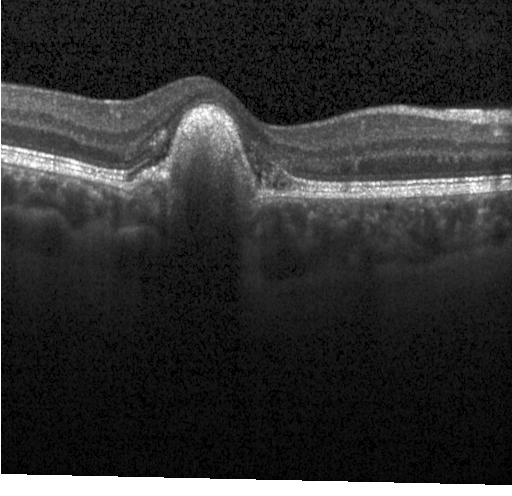
Optical coherence tomography B-scan; horizontal scan through the fovea; spectral-domain OCT; instrument: Heidelberg Spectralis.
Finding: a choroidal neovascular membrane.